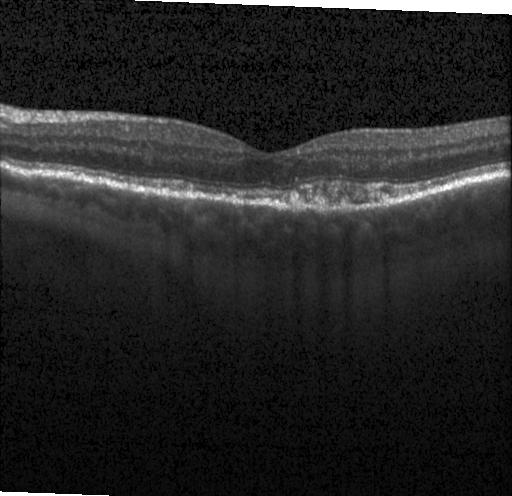 Optical coherence tomography scan · SD-OCT.
Macular OCT: sub-RPE drusenoid deposits.